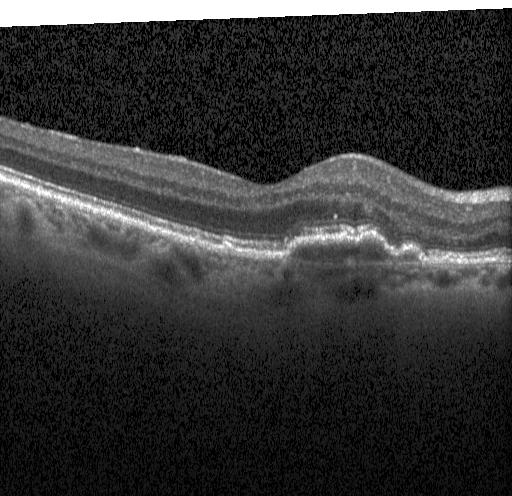

Optical coherence tomography B-scan; Heidelberg Spectralis OCT system; through the macula; SD-OCT — This B-scan demonstrates a choroidal neovascular membrane.